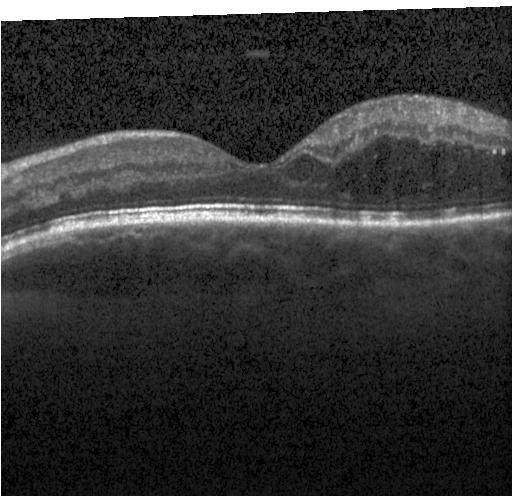 Macular OCT demonstrating DME.